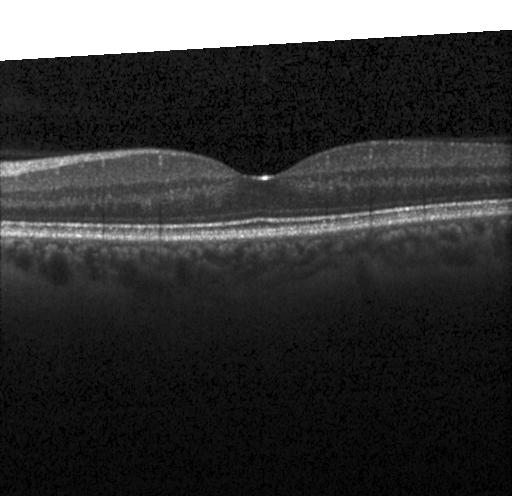 Spectral-domain OCT; retinal OCT cross-section; macular scan. Dx: no choroidal neovascularization, no diabetic macular edema, and no drusen.